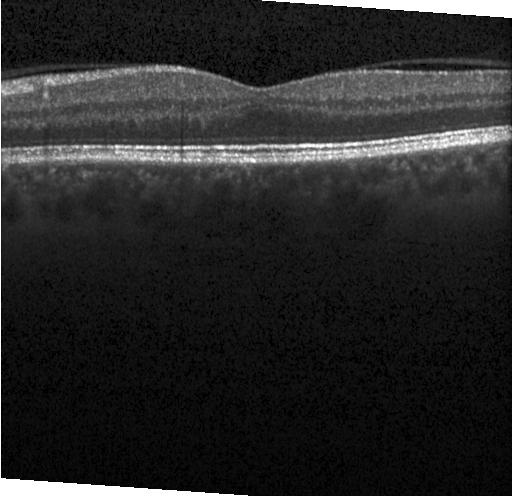

Heidelberg Spectralis · optical coherence tomography scan · macular scan — Impression: no choroidal neovascularization, diabetic macular edema, or drusen.